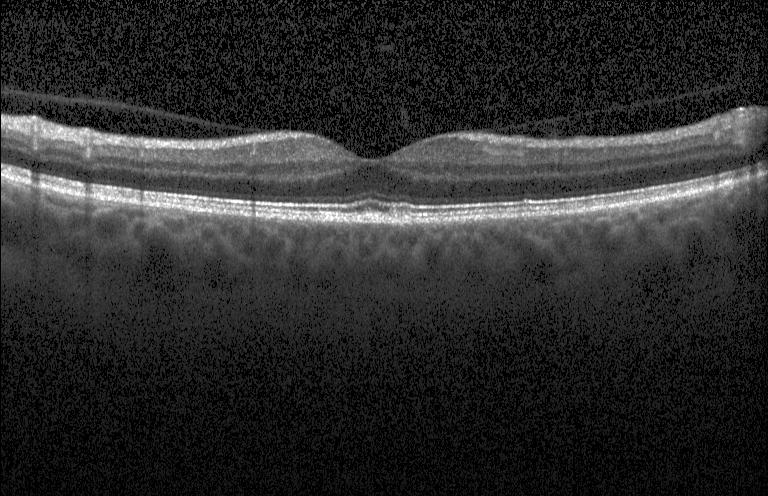
Retinal OCT cross-section. Spectral-domain optical coherence tomography. Instrument: Heidelberg Spectralis. The scan shows no CNV, no DME, and no drusen.